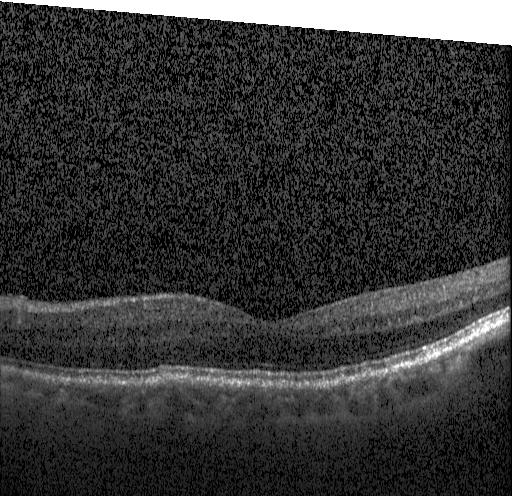
Diagnosis: no choroidal neovascularization, no diabetic macular edema, and no drusen.